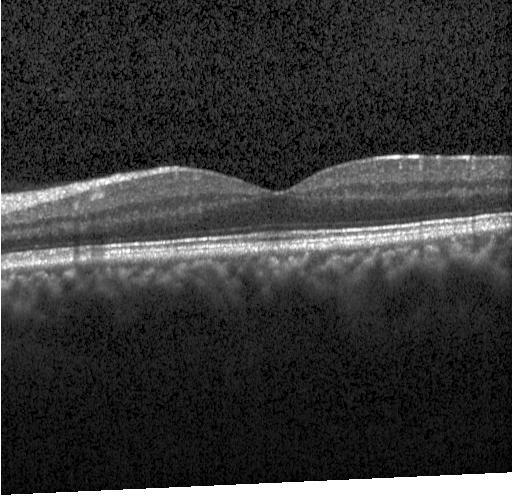

Heidelberg Spectralis. Spectral-domain optical coherence tomography. Retinal OCT cross-section — Assessment: no CNV, no DME, and no drusen.